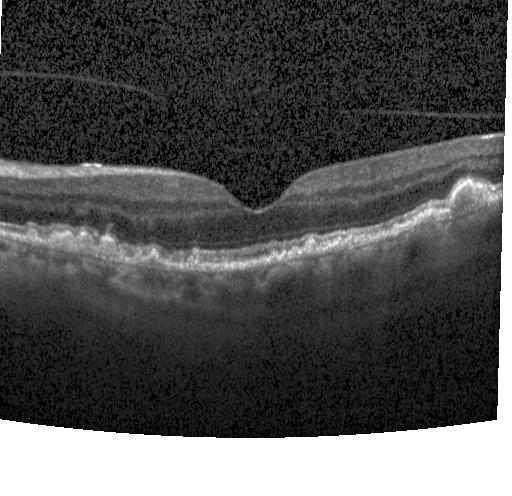

Spectral-domain optical coherence tomography · retinal OCT cross-section · Heidelberg Spectralis
Multiple drusen.